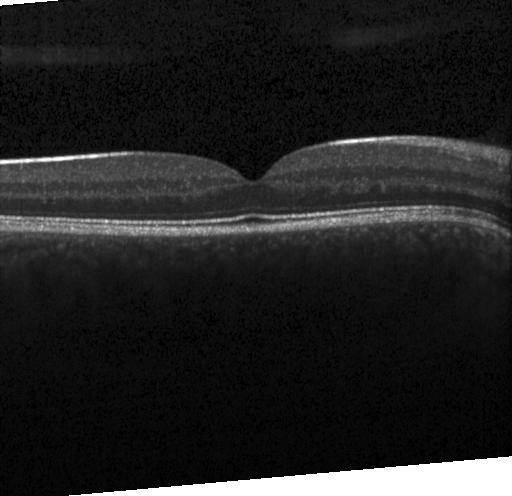

Optical coherence tomography B-scan
Diagnosis: neither choroidal neovascularization, diabetic macular edema, nor drusen.